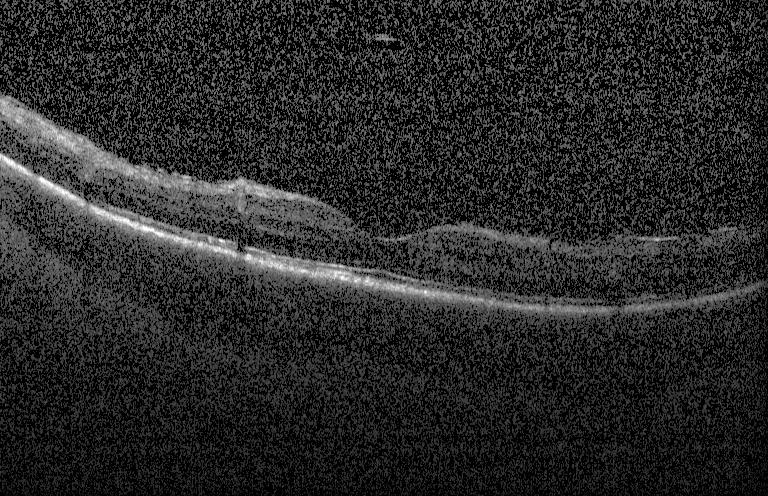 Finding: no CNV, no DME, and no drusen.